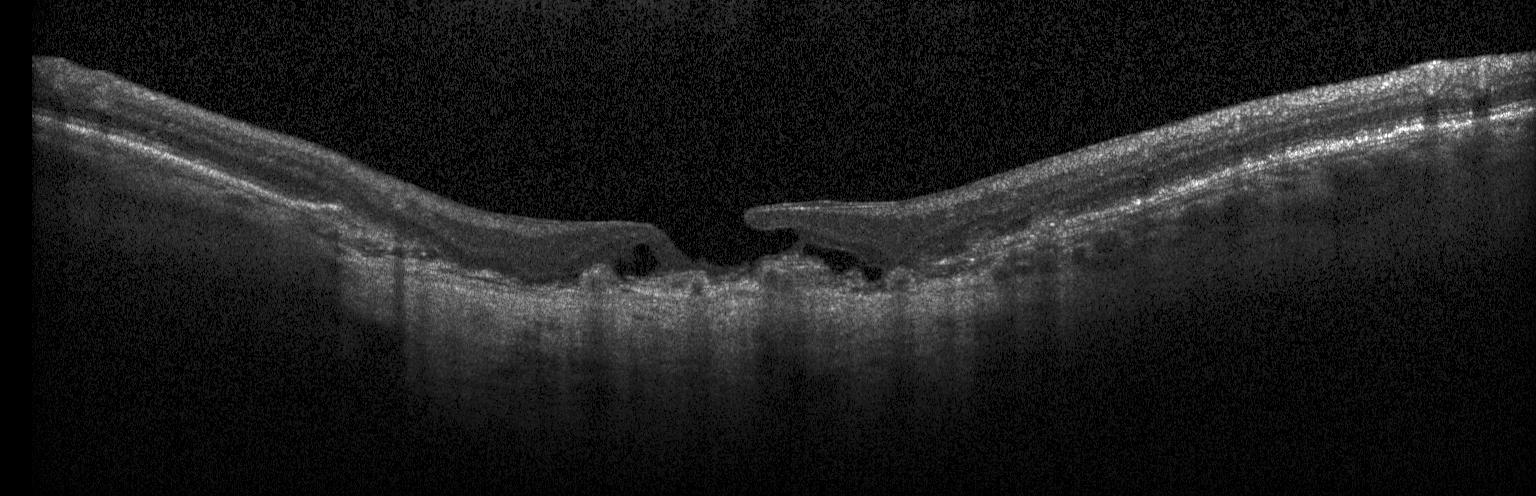

Spectral-domain optical coherence tomography · OCT line scan · macular scan · instrument: Heidelberg Spectralis
Diagnosis: choroidal neovascularization (CNV).